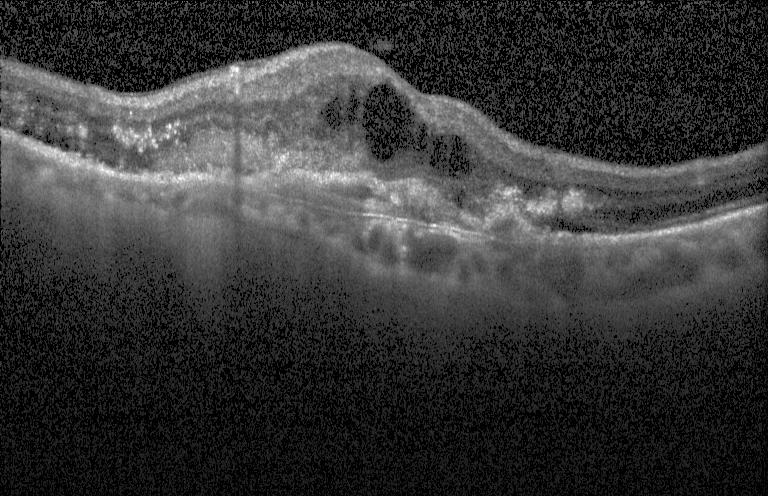 Diagnosis: CNV.